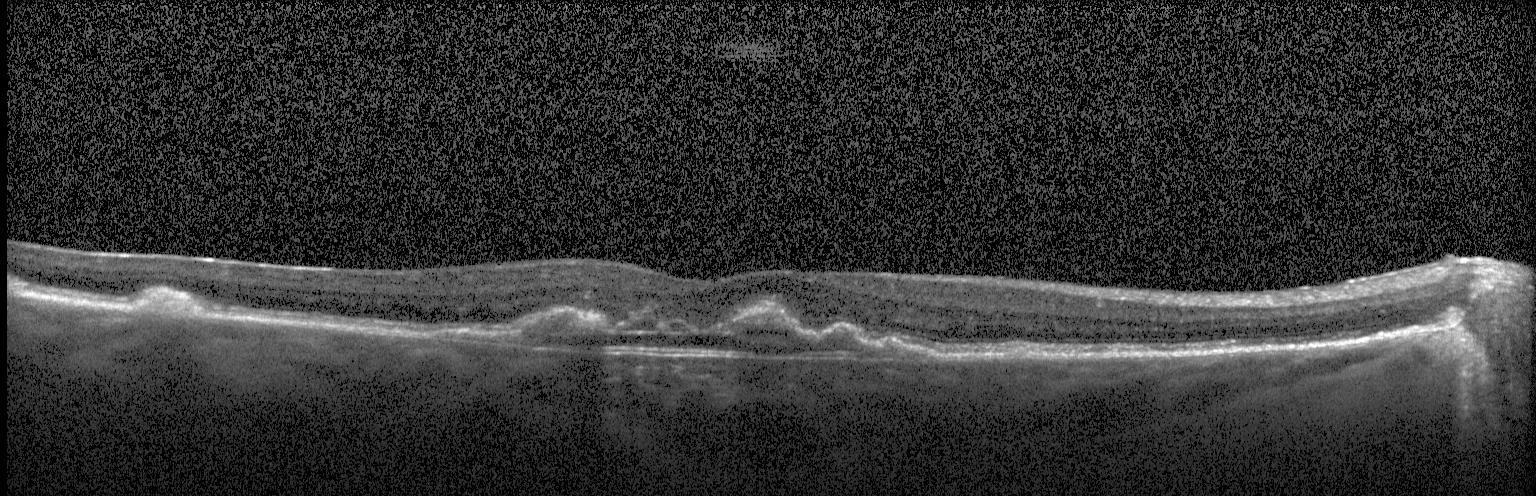

Optical coherence tomography B-scan, spectral-domain optical coherence tomography, instrument: Heidelberg Spectralis
Finding: a choroidal neovascular membrane.